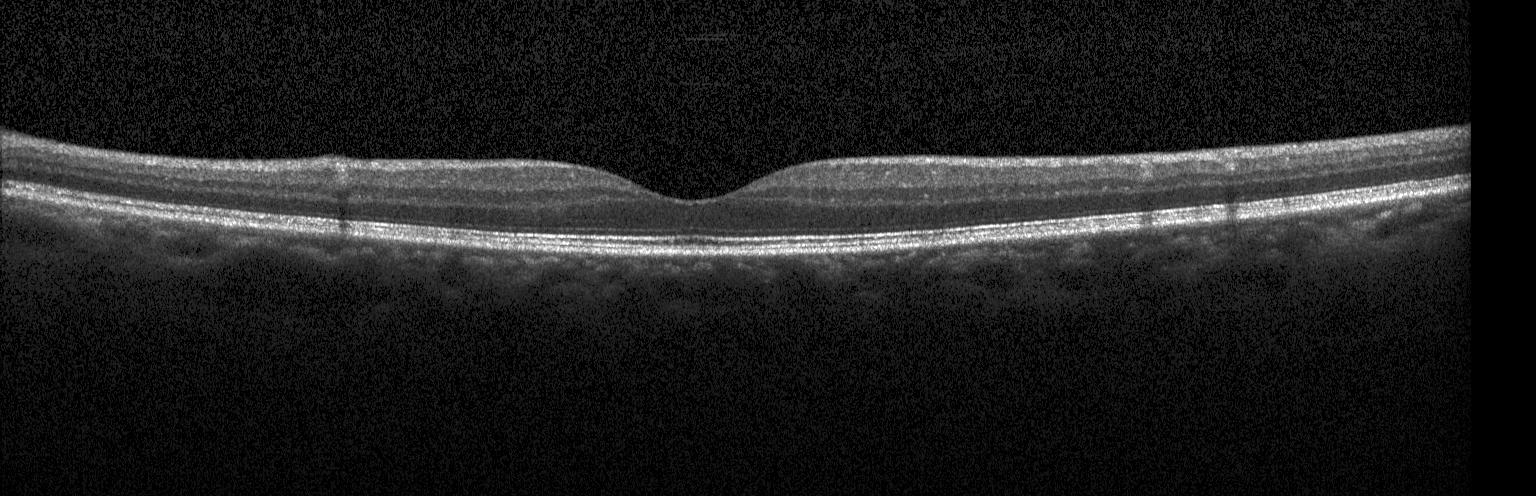
Macular OCT demonstrating no choroidal neovascularization, diabetic macular edema, or drusen.